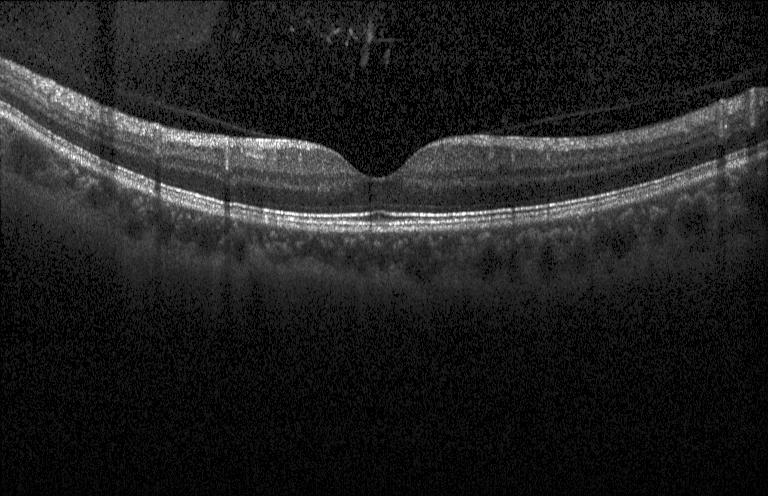

Retinal OCT B-scan — This B-scan demonstrates no choroidal neovascularization, diabetic macular edema, or drusen.